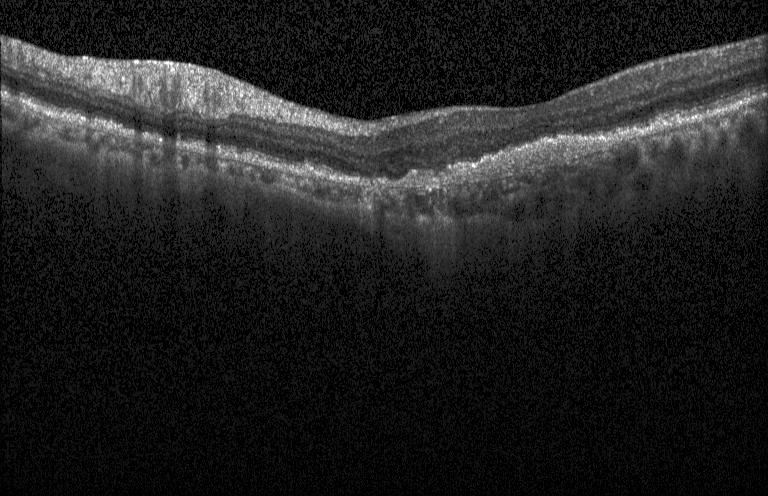
Diagnosis: choroidal neovascularization (CNV).